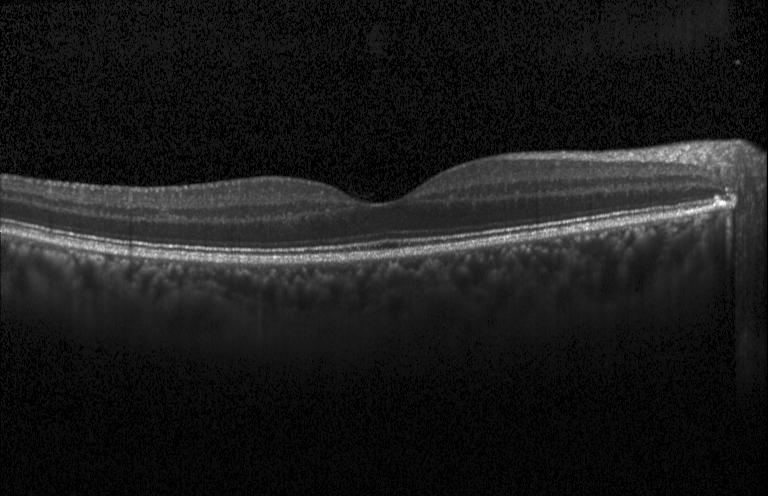
Finding: neither CNV, DME, nor drusen.